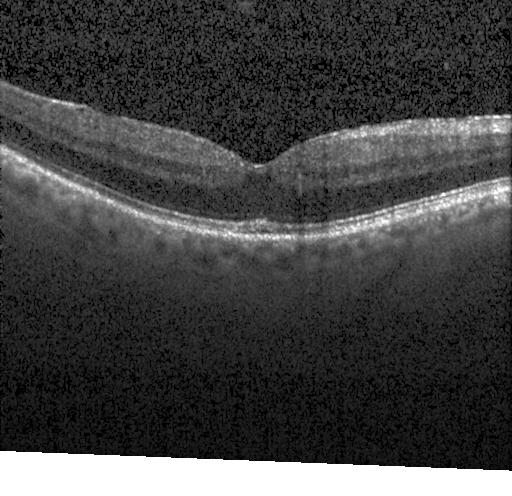
Horizontal scan through the fovea; retinal OCT B-scan. Assessment: neither CNV, DME, nor drusen.